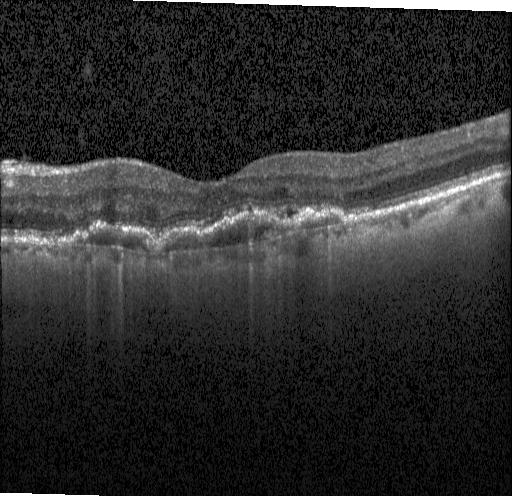
This B-scan demonstrates choroidal neovascularization.